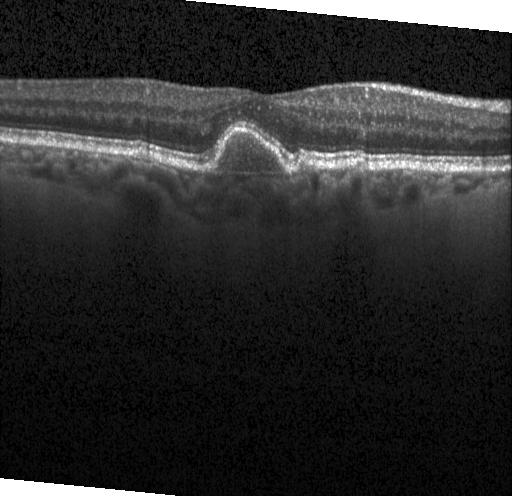

Retinal OCT cross-section, fovea-centered, Heidelberg Spectralis — Impression: a choroidal neovascular membrane.